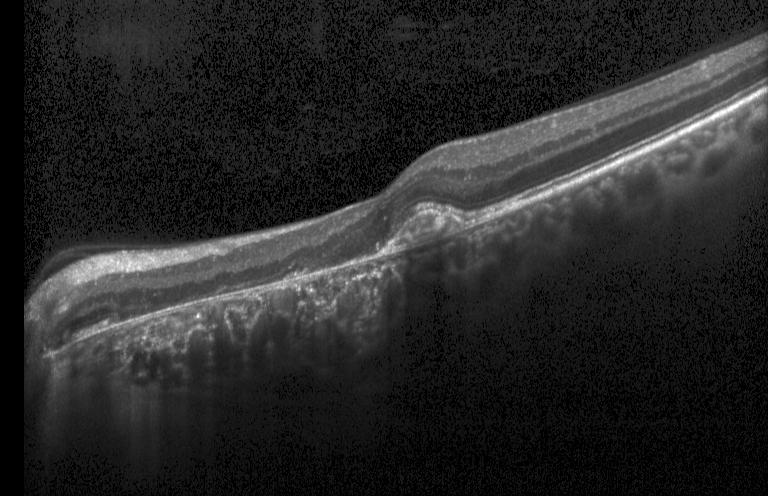

Finding: choroidal neovascularization (CNV).